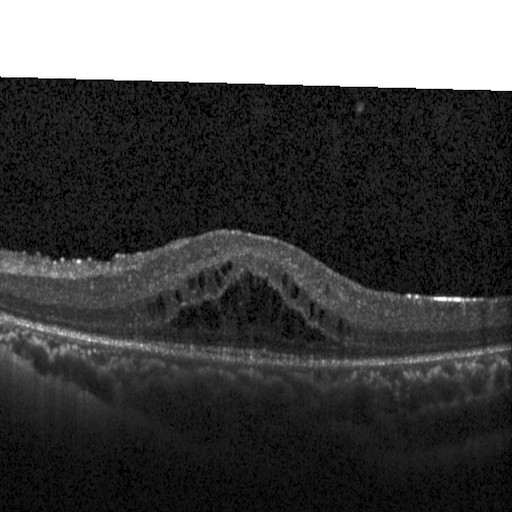

Optical coherence tomography B-scan; Heidelberg Spectralis OCT system
Diagnosis: DME.